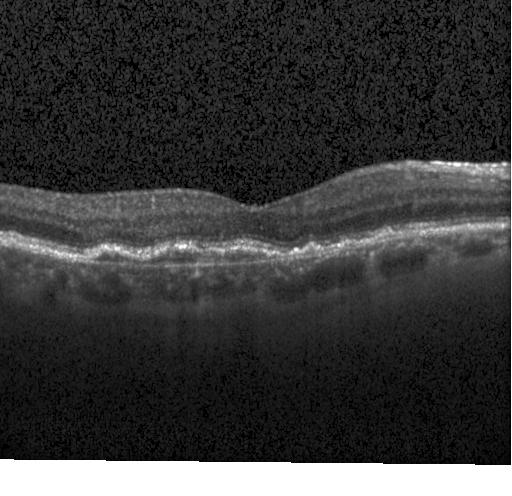

This B-scan demonstrates a choroidal neovascular membrane.